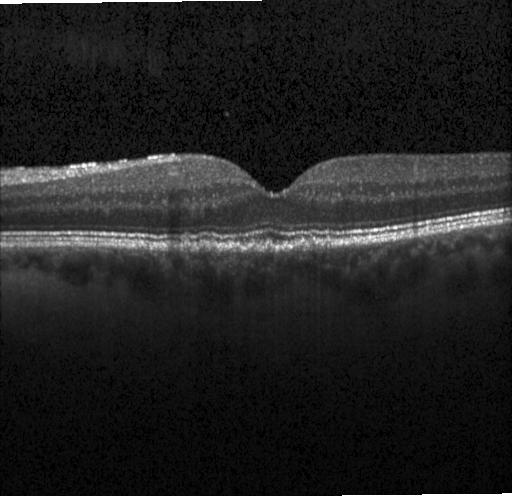
Macular OCT: sub-RPE drusenoid deposits.